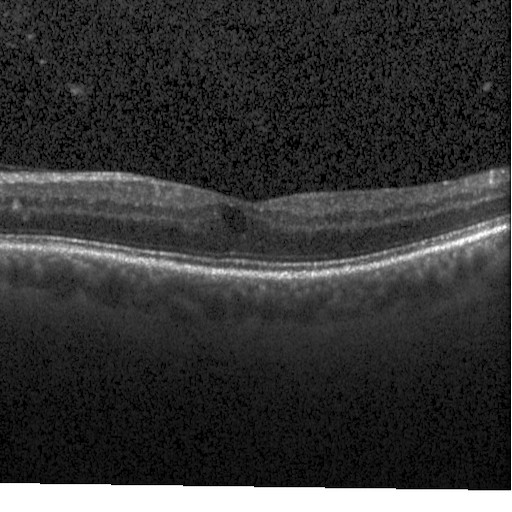
Retinal OCT B-scan; acquired on a Heidelberg Spectralis. Finding: DME.